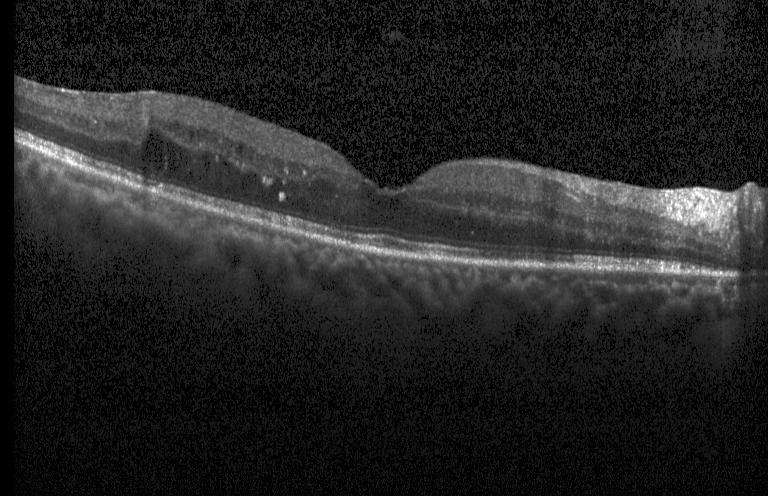

OCT line scan.
The scan shows diabetic macular edema.